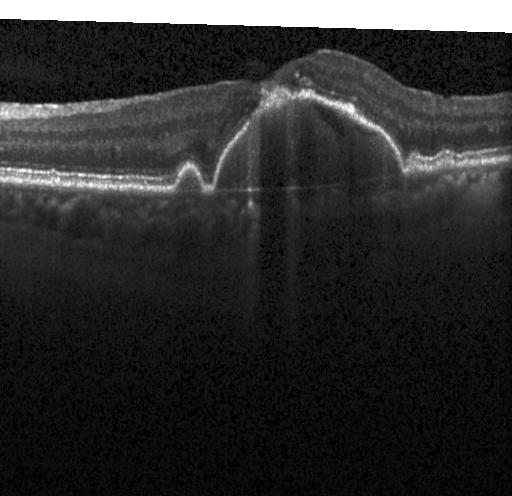 Retinal OCT cross-section. Diagnosis: a choroidal neovascular membrane.